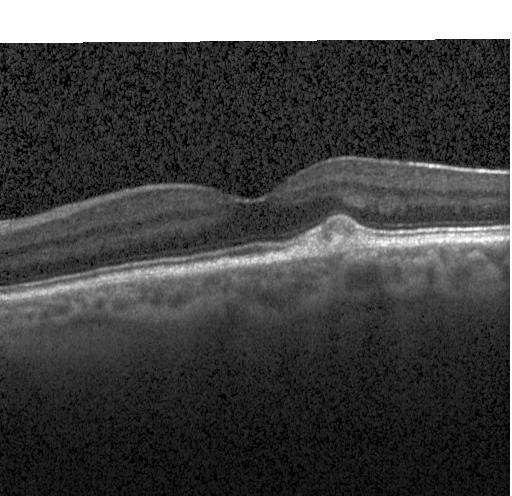

Instrument: Heidelberg Spectralis; fovea-centered; spectral-domain optical coherence tomography; OCT B-scan — Impression: drusen.